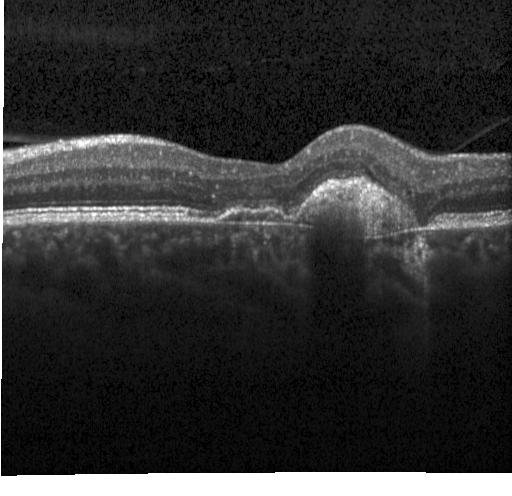

Optical coherence tomography scan; instrument: Heidelberg Spectralis — Finding: a choroidal neovascular membrane.